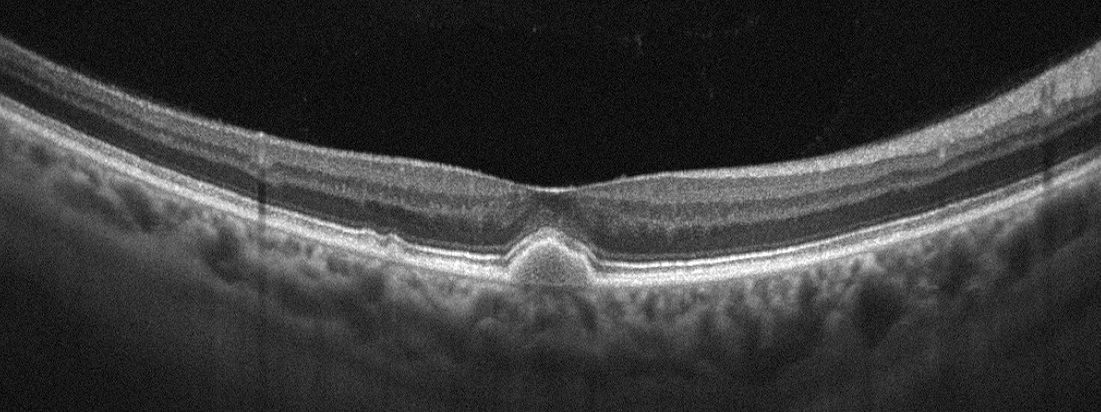

Optical coherence tomography B-scan. Macular scan
The scan shows age-related macular degeneration.